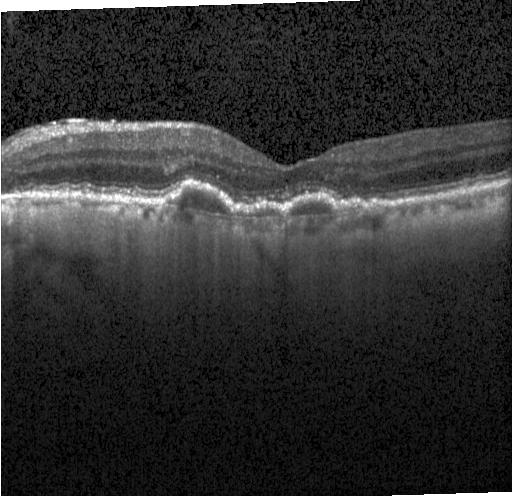
Dx: CNV.